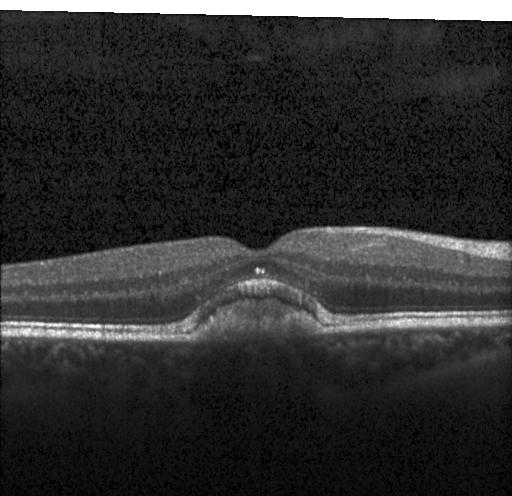 Retinal OCT cross-section. Through the macula. Heidelberg Spectralis OCT system
Diagnosis: a choroidal neovascular membrane.